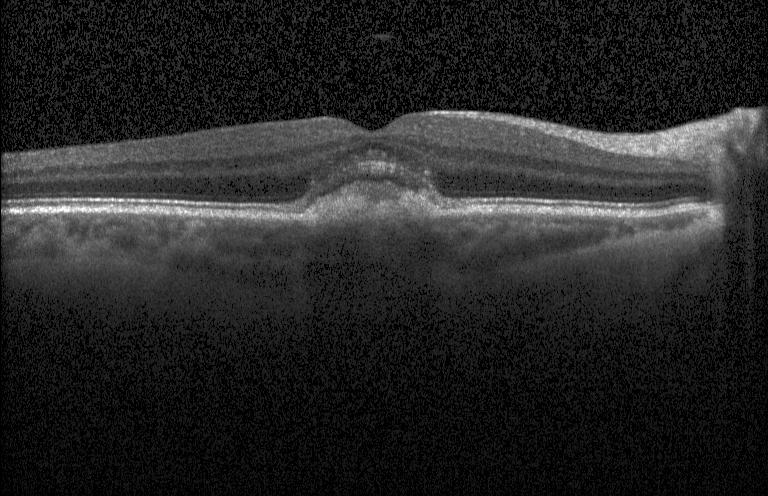
Retinal OCT B-scan
Diagnosis: a choroidal neovascular membrane.